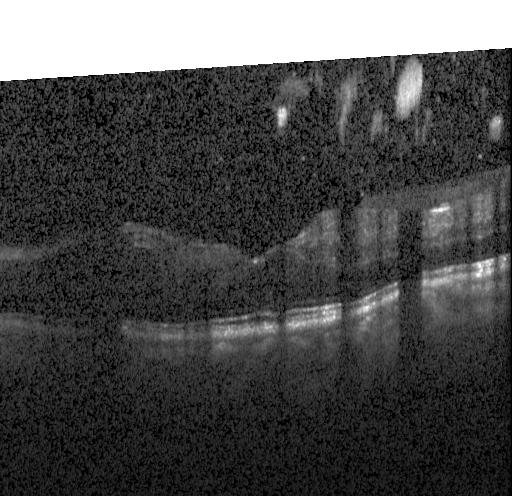
The scan shows no evidence of CNV, DME, or drusen.